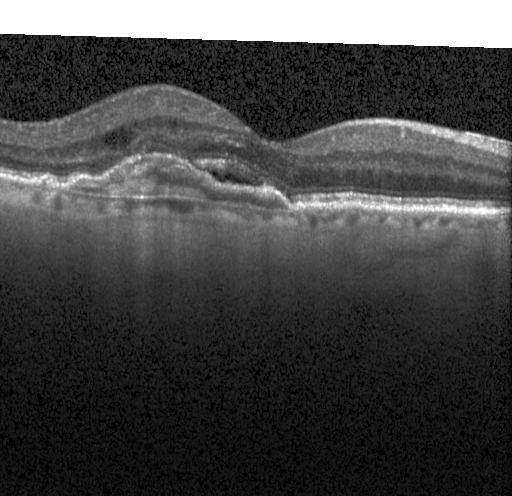

Instrument: Heidelberg Spectralis. Optical coherence tomography B-scan. SD-OCT. Horizontal scan through the fovea — Diagnosis: a choroidal neovascular membrane.